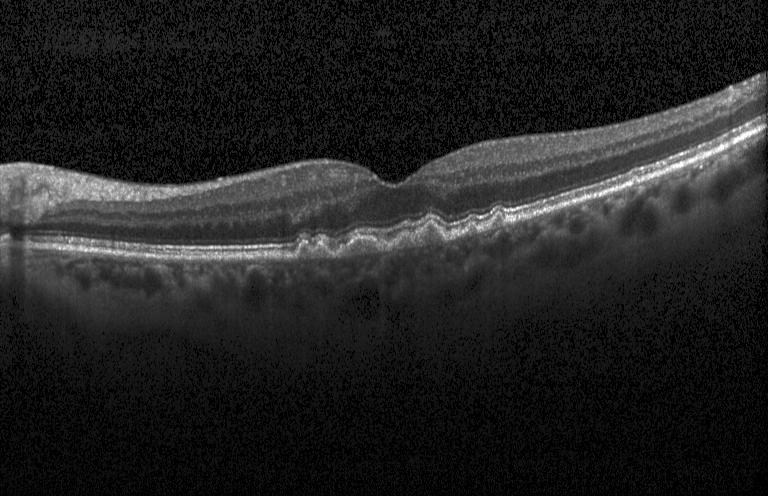

Macular OCT: sub-RPE drusenoid deposits.